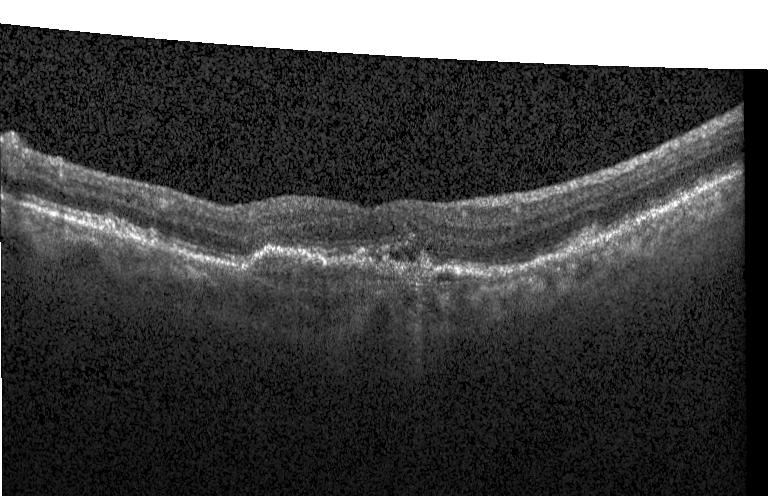
Retinal OCT B-scan. Heidelberg Spectralis. SD-OCT. Through the macula — Finding: choroidal neovascularization (CNV).